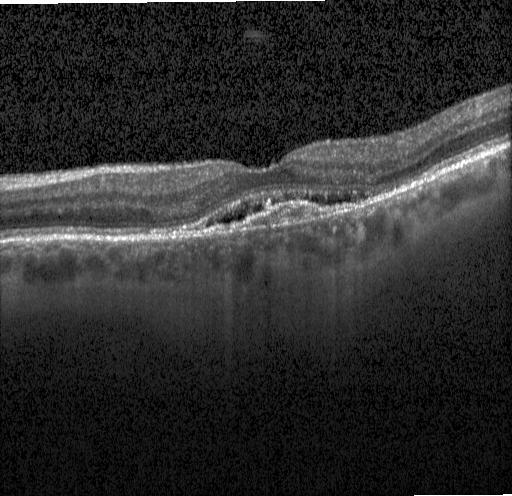

Retinal OCT cross-section showing a choroidal neovascular membrane.